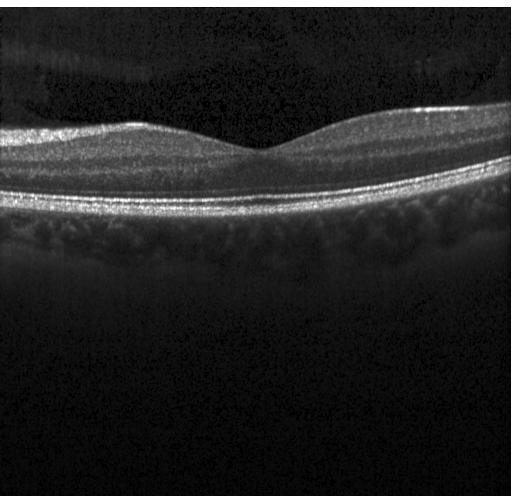

OCT finding: no evidence of choroidal neovascularization, diabetic macular edema, or drusen.